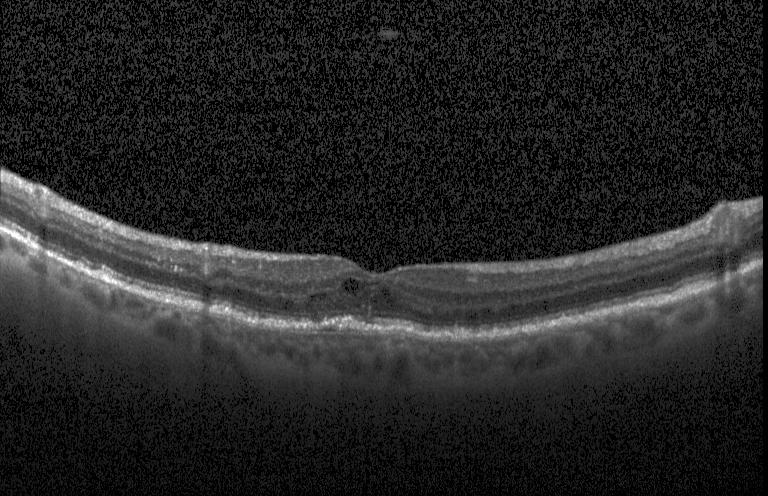 Diagnosis: a choroidal neovascular membrane.